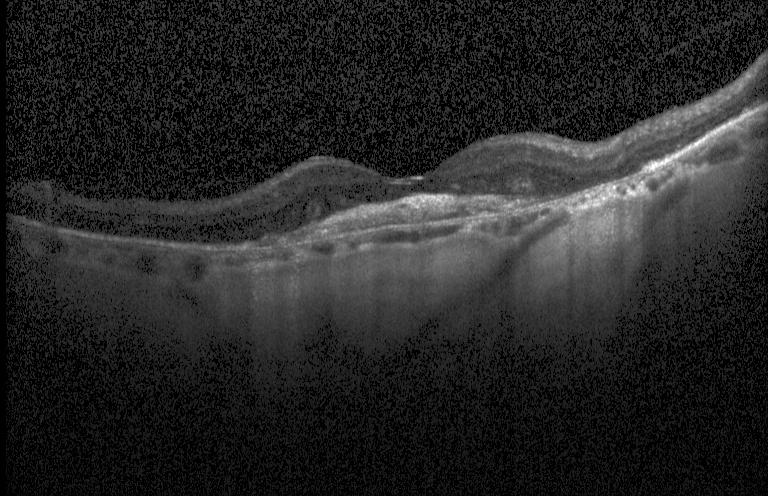 Diagnosis: choroidal neovascularization (CNV).